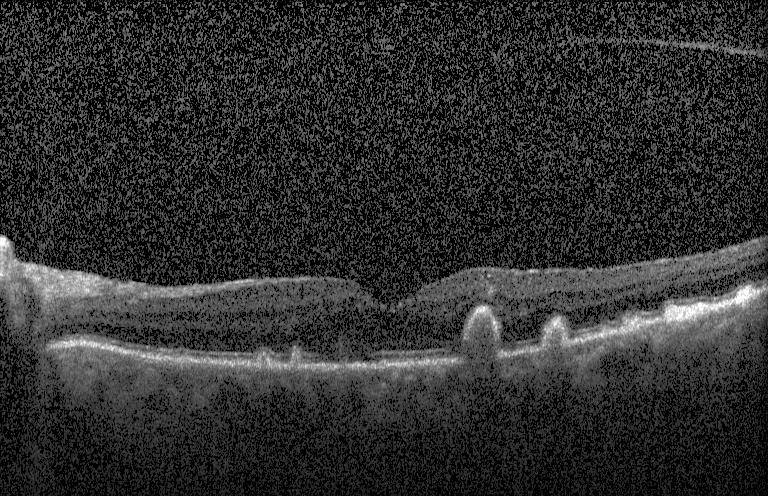
Retinal OCT cross-section; acquired on a Heidelberg Spectralis; macular scan; SD-OCT. Assessment: sub-RPE drusenoid deposits.